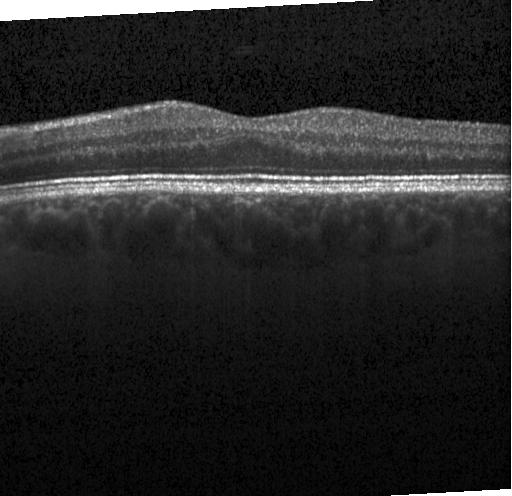 Assessment: no CNV, no DME, and no drusen.